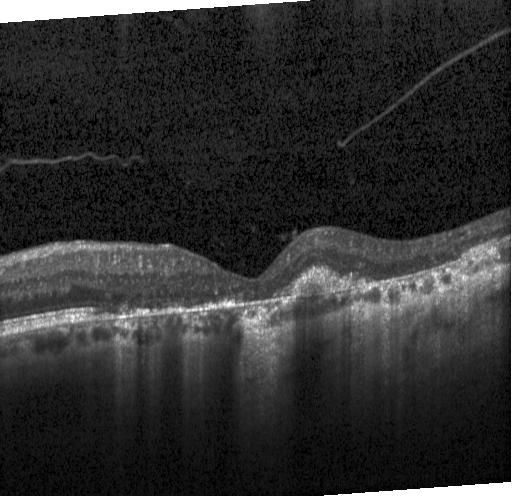
OCT finding: a choroidal neovascular membrane.